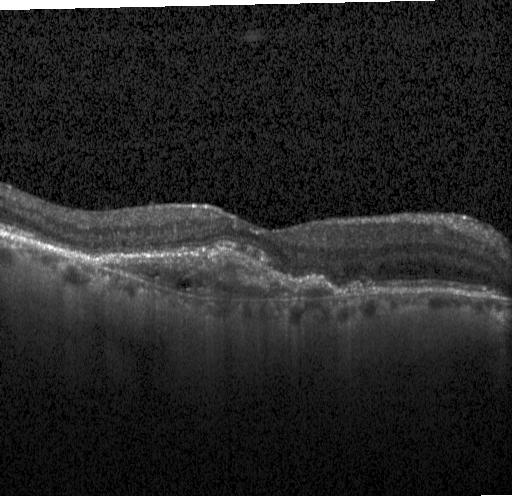 Retinal OCT cross-section showing a choroidal neovascular membrane.